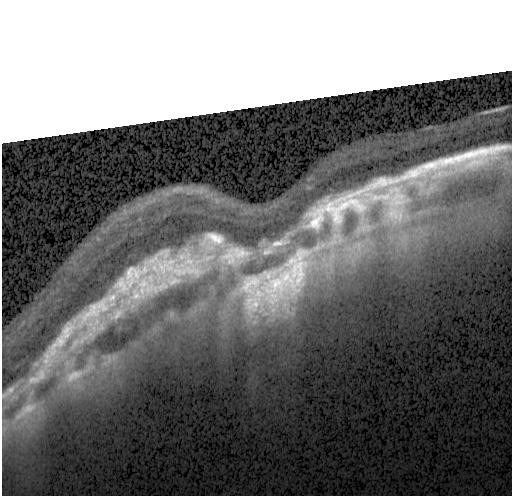 Retinal OCT B-scan
OCT finding: a choroidal neovascular membrane.